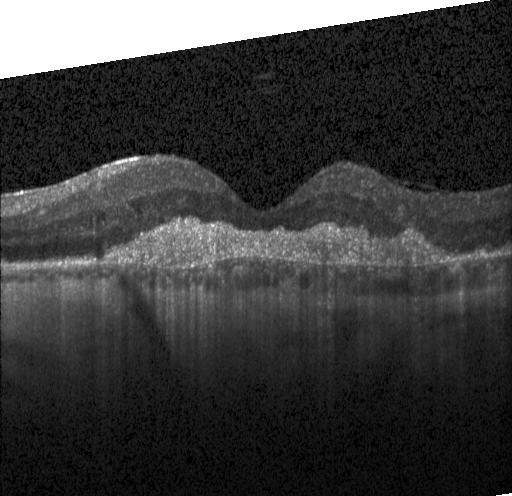
The scan shows choroidal neovascularization.